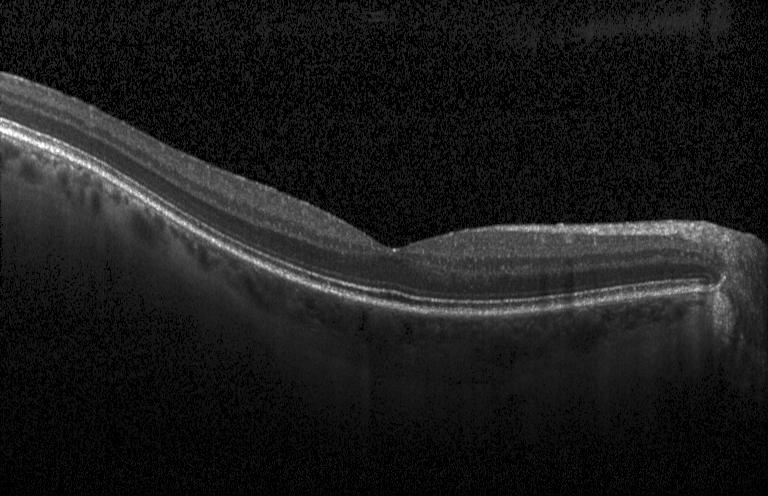

Fovea-centered. OCT B-scan. The scan shows neither CNV, DME, nor drusen.